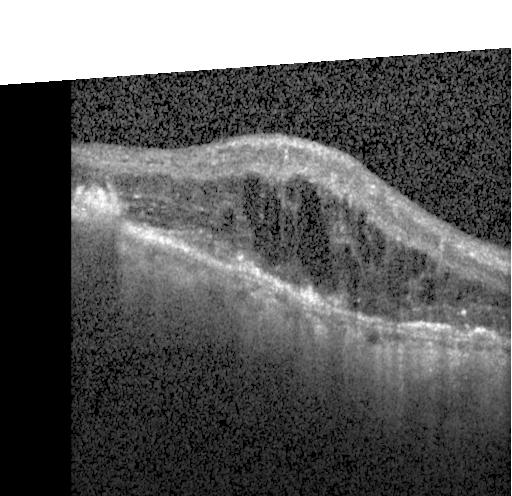 A choroidal neovascular membrane.